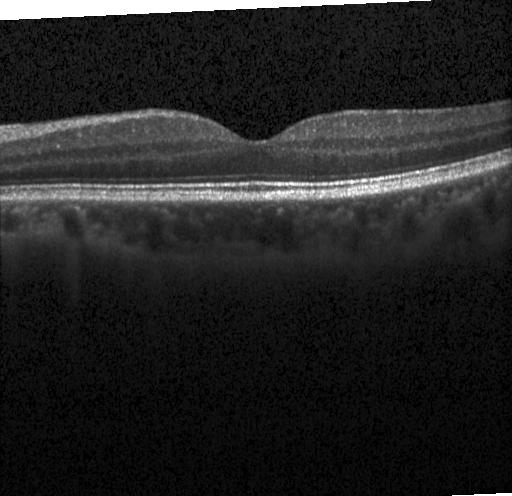 Retinal OCT B-scan, fovea-centered
Assessment: no choroidal neovascularization, no diabetic macular edema, and no drusen.